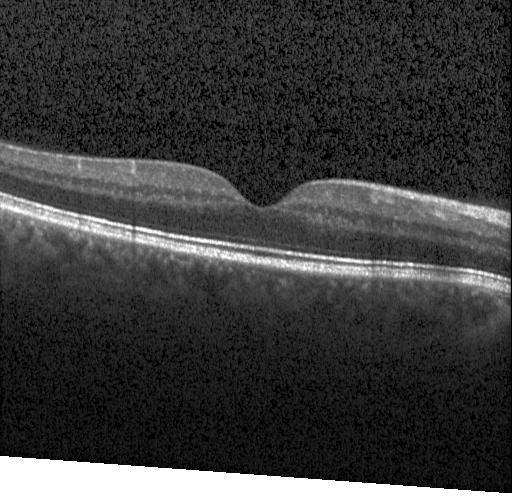
Heidelberg Spectralis OCT system · spectral-domain optical coherence tomography · optical coherence tomography scan. The scan shows no choroidal neovascularization, no diabetic macular edema, and no drusen.